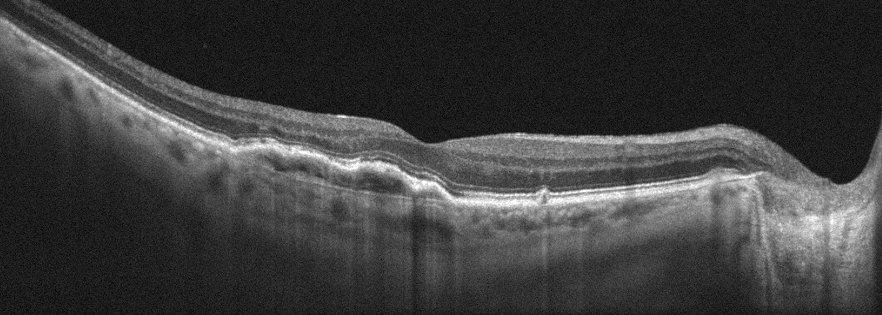
Optical coherence tomography scan. Instrument: Optovue Avanti RTVue XR. OD. Through the macula. Diagnosis: AMD.